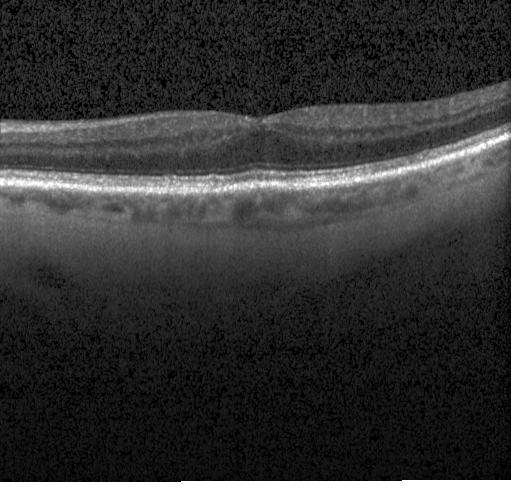 Macular OCT: no evidence of CNV, DME, or drusen.